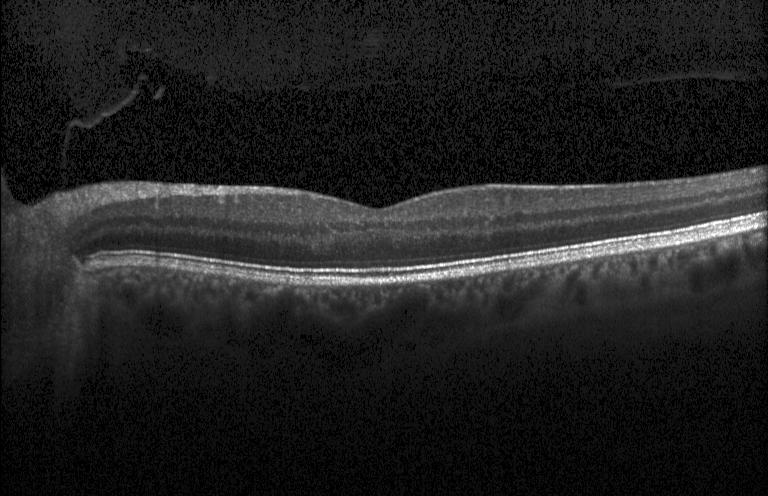

Finding: neither choroidal neovascularization, diabetic macular edema, nor drusen.